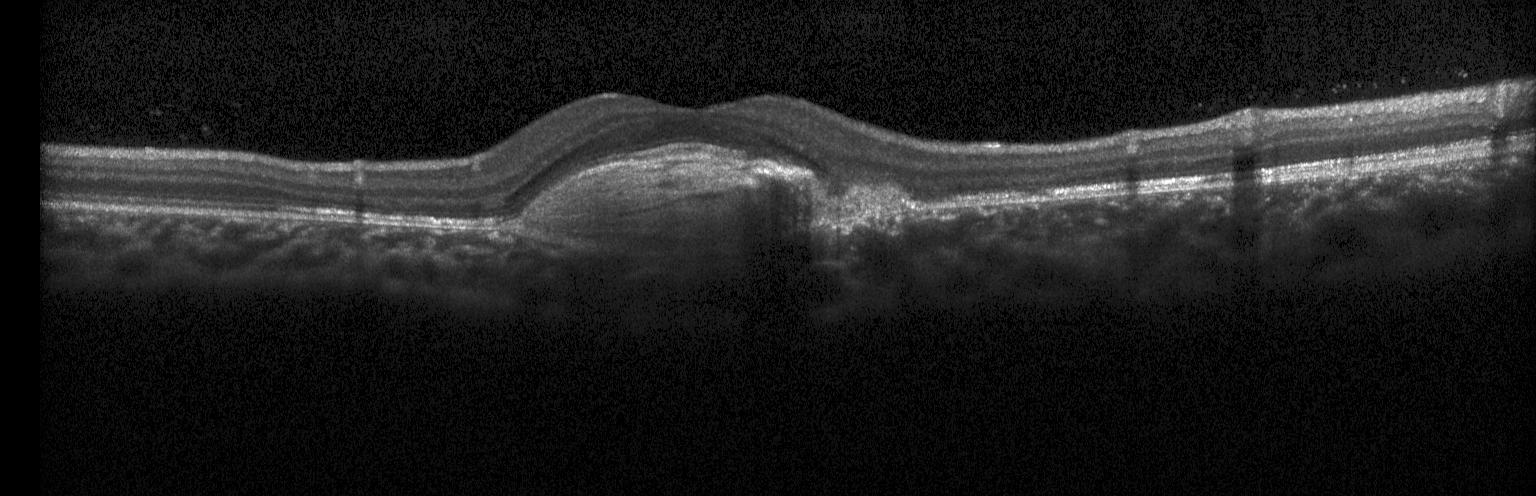

Macular OCT: a choroidal neovascular membrane.